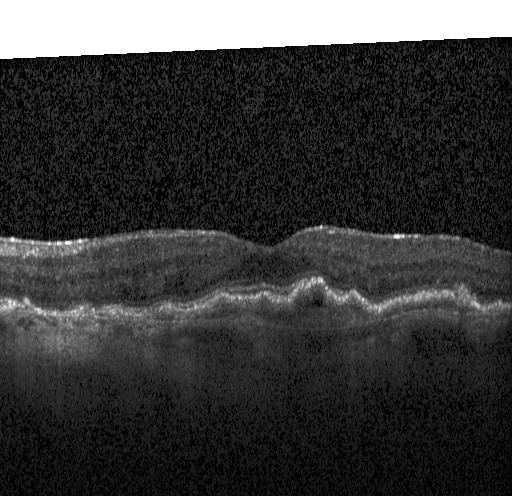 Heidelberg Spectralis OCT system · spectral-domain OCT · macular scan · optical coherence tomography B-scan. The scan shows a choroidal neovascular membrane.